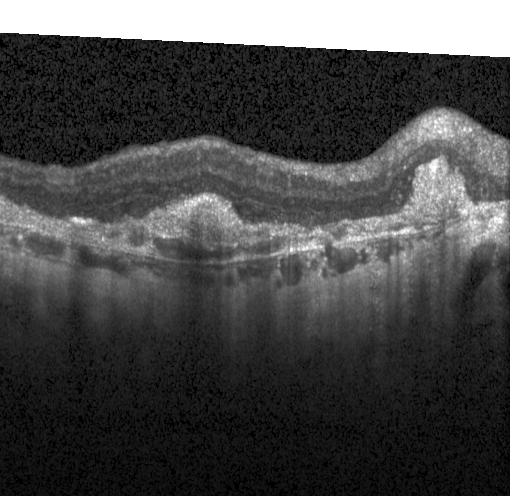
A choroidal neovascular membrane.